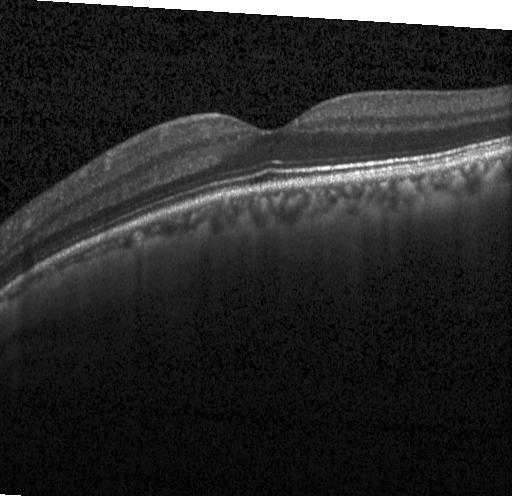 Spectral-domain OCT · Heidelberg Spectralis · macular scan · optical coherence tomography B-scan.
Impression: no CNV, DME, or drusen.